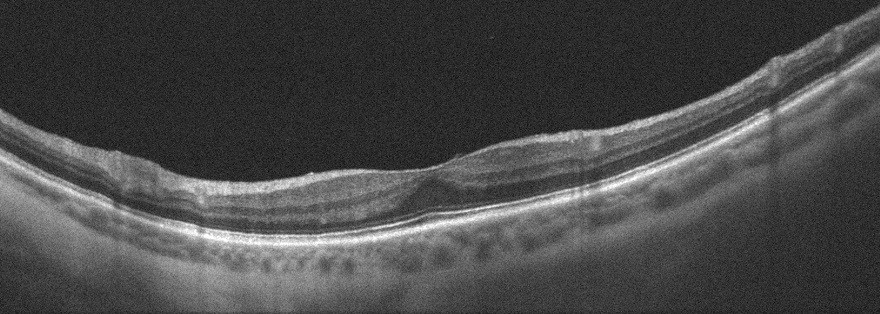 Macular scan. Retinal OCT B-scan
Finding: ERM.